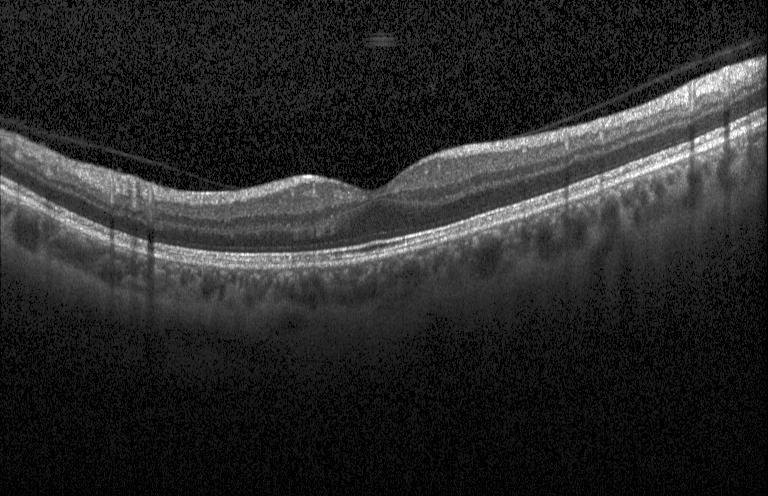

Optical coherence tomography B-scan · SD-OCT · horizontal scan through the fovea.
This B-scan demonstrates neither choroidal neovascularization, diabetic macular edema, nor drusen.